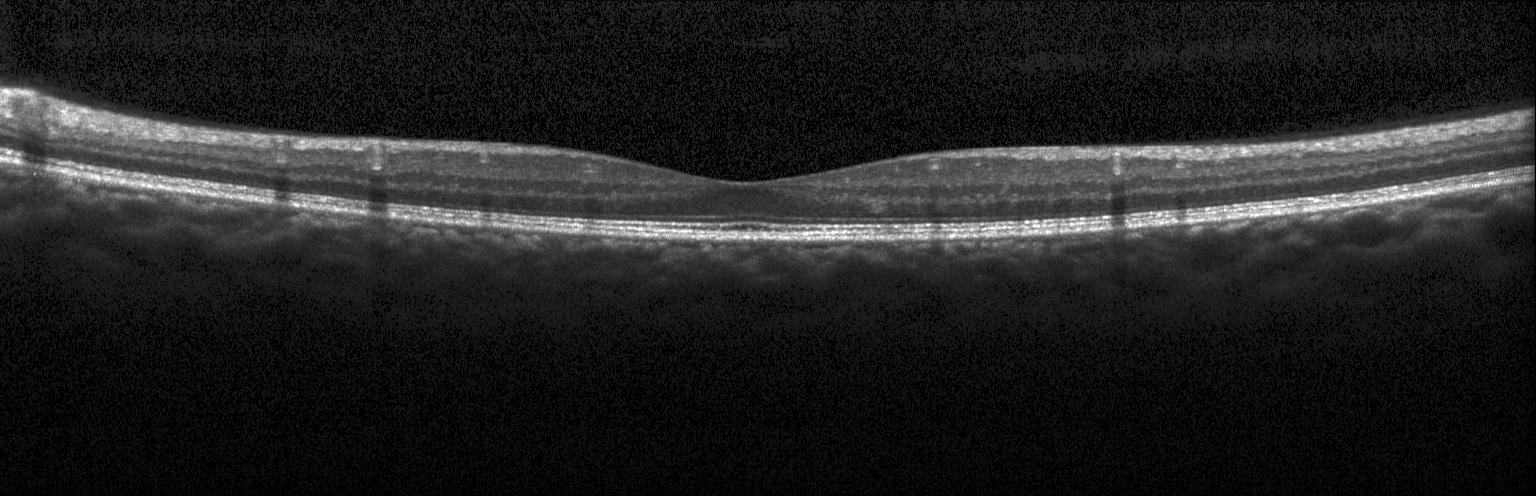

Retinal OCT cross-section showing no CNV, no DME, and no drusen.